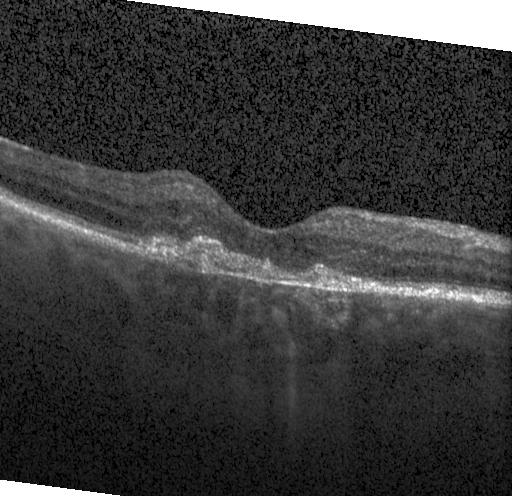

Impression: choroidal neovascularization.